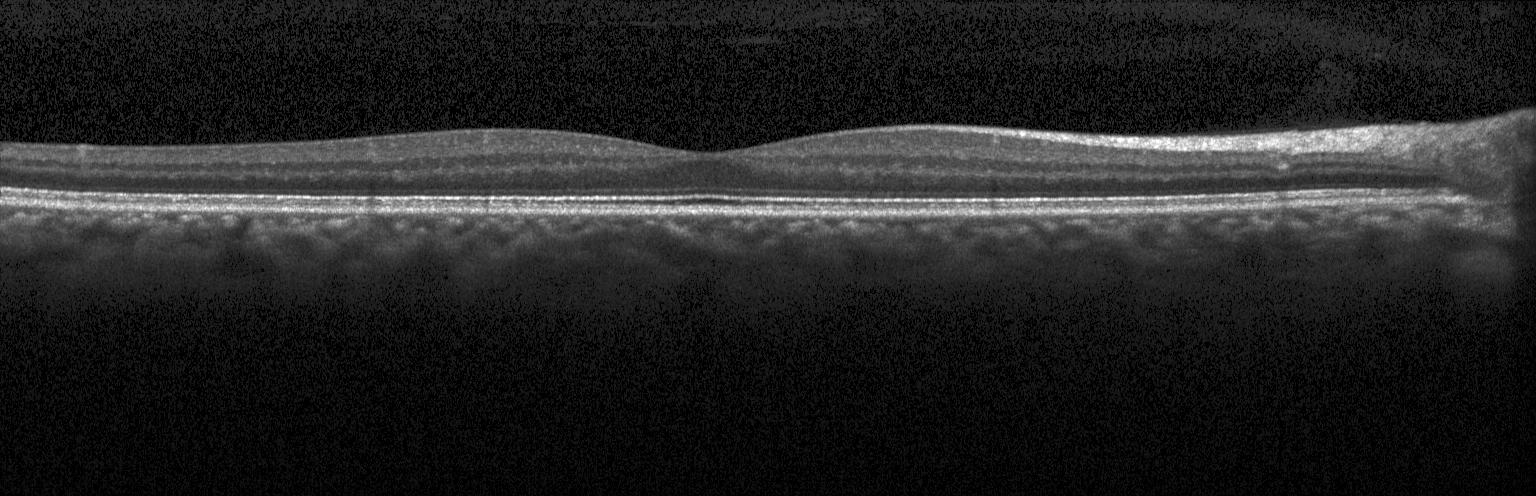 OCT finding: neither choroidal neovascularization, diabetic macular edema, nor drusen.